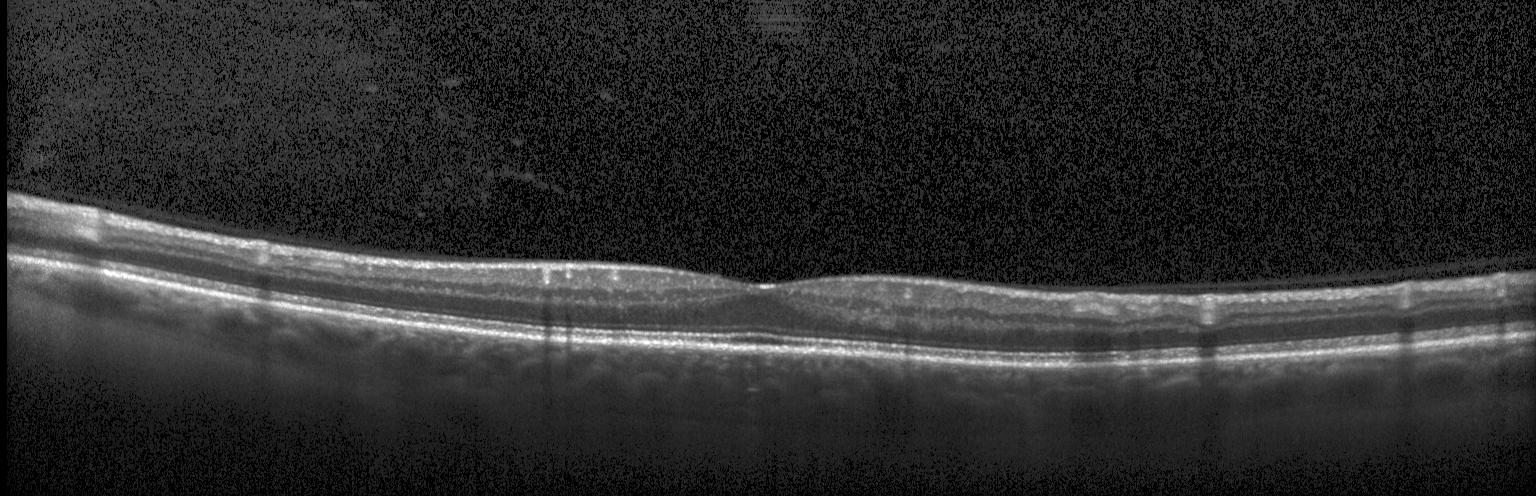 Heidelberg Spectralis OCT system; OCT line scan; spectral-domain optical coherence tomography; centered on the fovea.
No CNV, no DME, and no drusen.